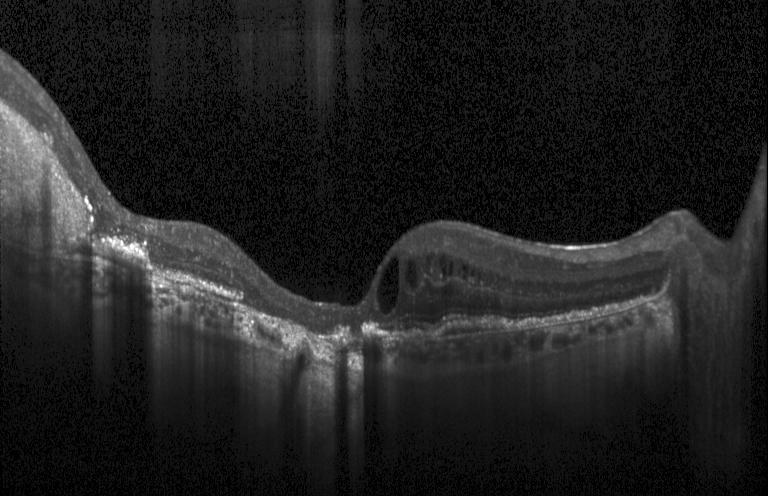 Spectral-domain OCT B-scan: a choroidal neovascular membrane.